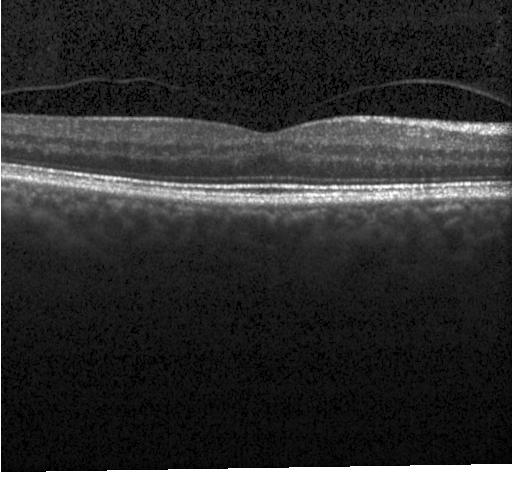
Finding: no evidence of choroidal neovascularization, diabetic macular edema, or drusen.